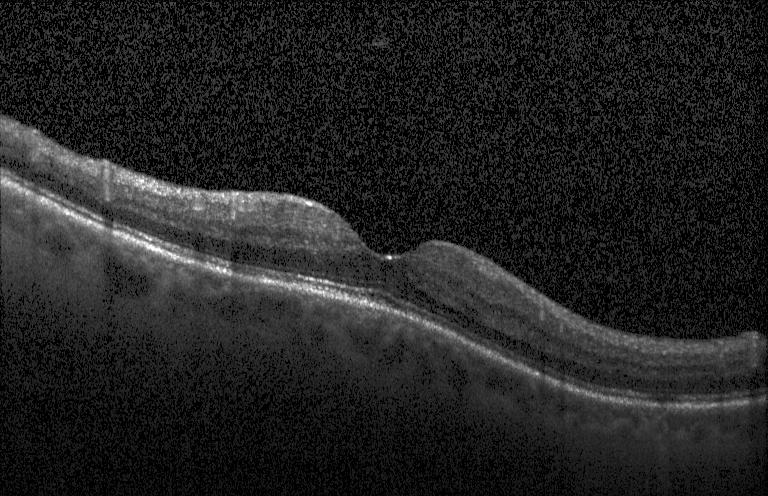

Optical coherence tomography scan. Through the macula
No choroidal neovascularization, diabetic macular edema, or drusen.